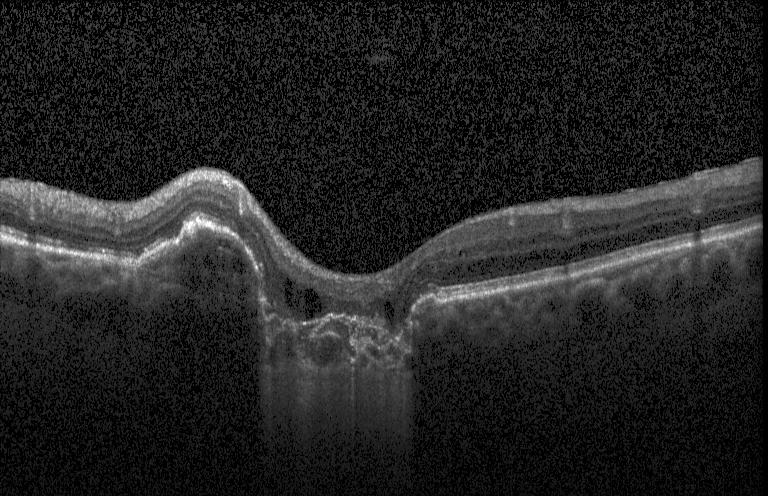

Instrument: Heidelberg Spectralis. OCT line scan. Finding: CNV.